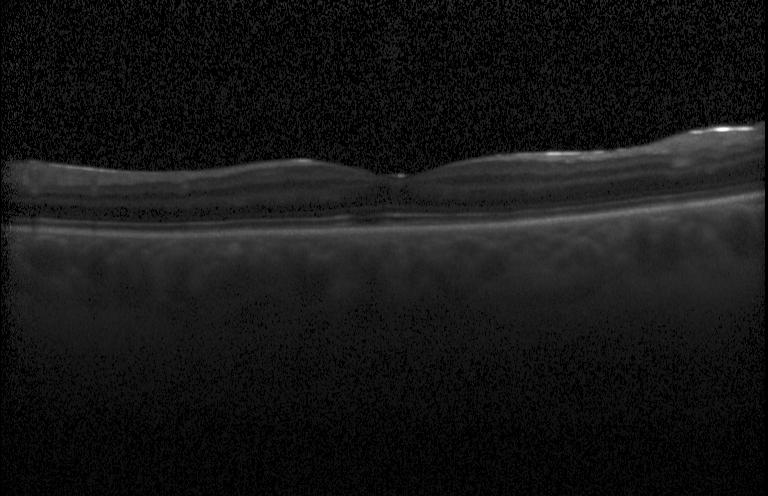 Spectral-domain OCT B-scan: no evidence of CNV, DME, or drusen.